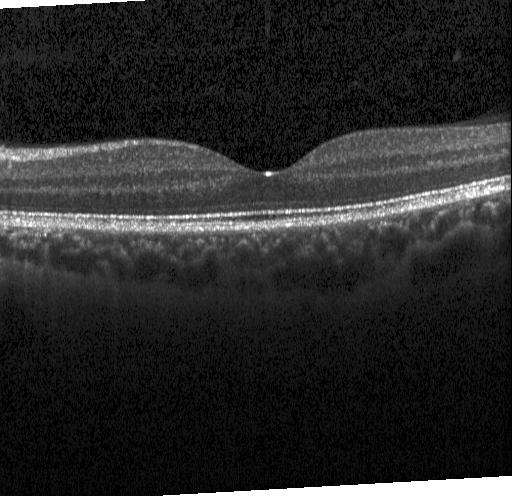

Optical coherence tomography scan; centered on the fovea; acquired on a Heidelberg Spectralis; spectral-domain optical coherence tomography — This B-scan demonstrates no choroidal neovascularization, no diabetic macular edema, and no drusen.